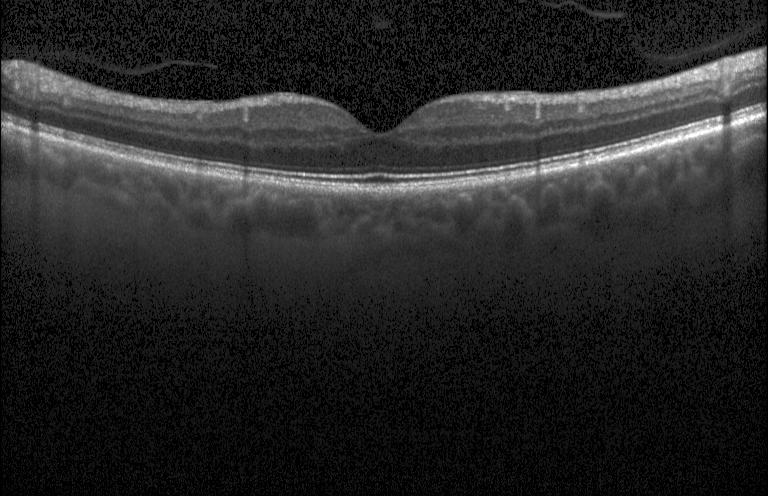
Acquired on a Heidelberg Spectralis. SD-OCT. Optical coherence tomography B-scan. Centered on the fovea
Impression: no CNV, DME, or drusen.